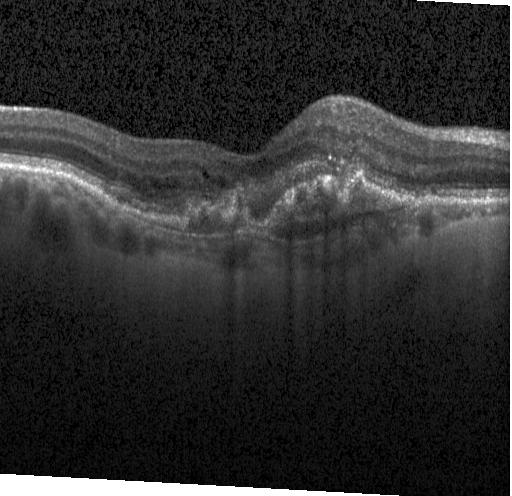 Retinal OCT cross-section.
This B-scan demonstrates a choroidal neovascular membrane.